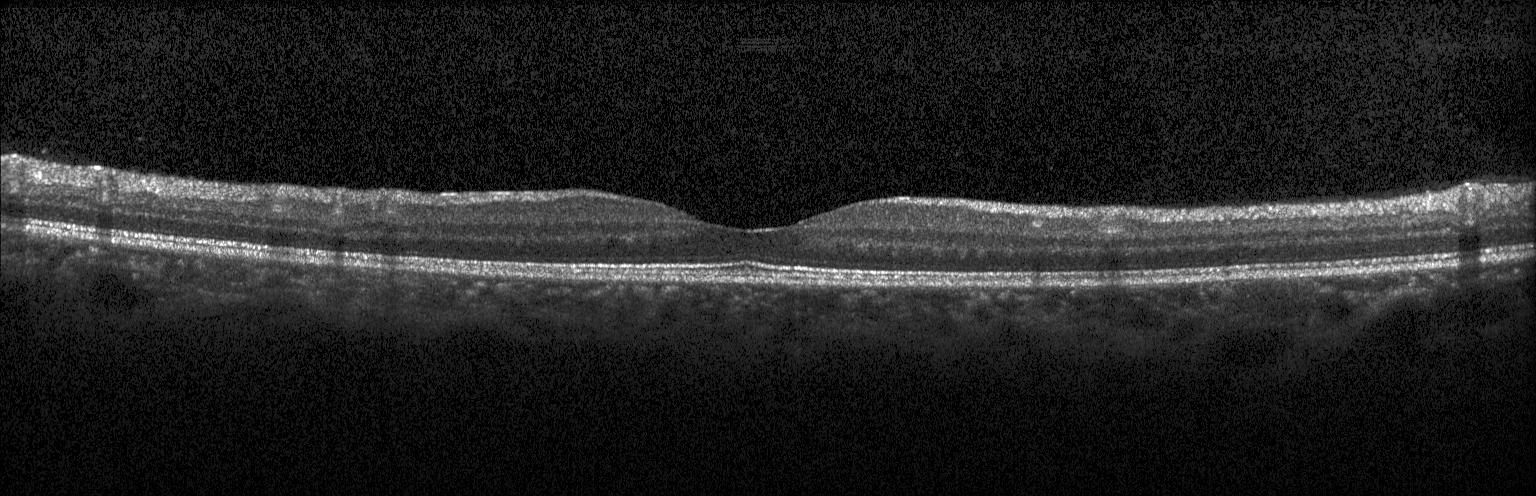

Finding: neither choroidal neovascularization, diabetic macular edema, nor drusen.